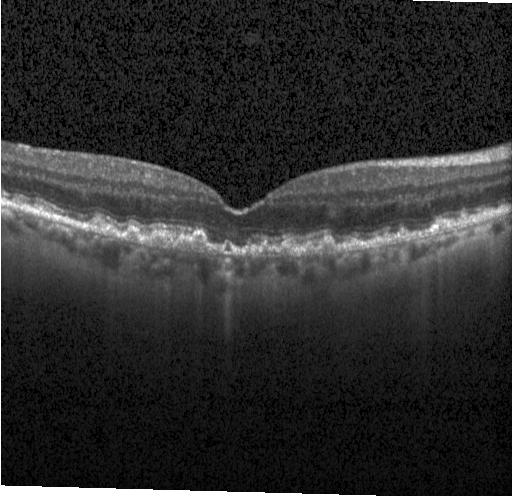 Optical coherence tomography B-scan. Instrument: Heidelberg Spectralis — The scan shows sub-RPE drusenoid deposits.